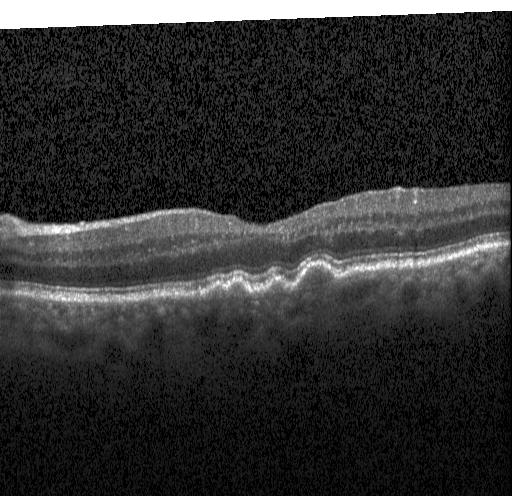
Macular OCT: multiple drusen.